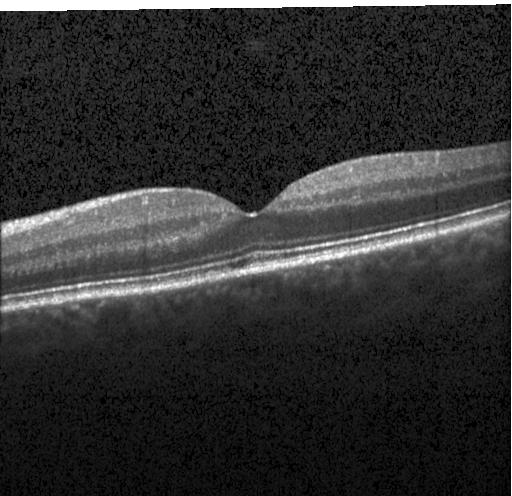

Diagnosis: neither choroidal neovascularization, diabetic macular edema, nor drusen.